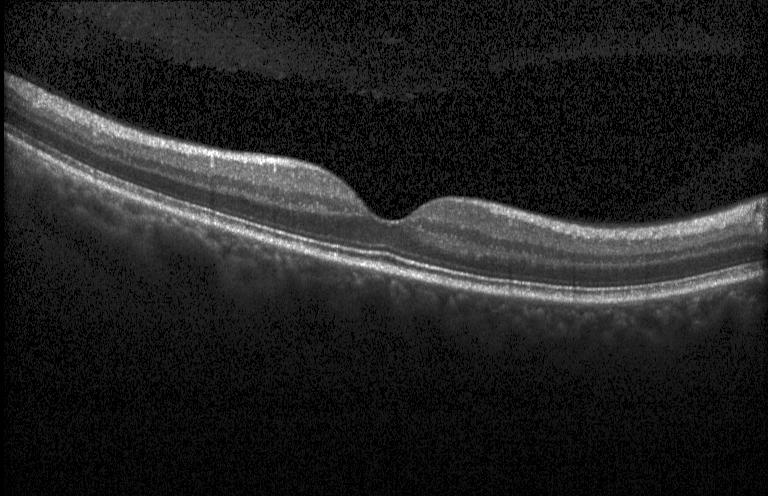 No choroidal neovascularization, no diabetic macular edema, and no drusen.